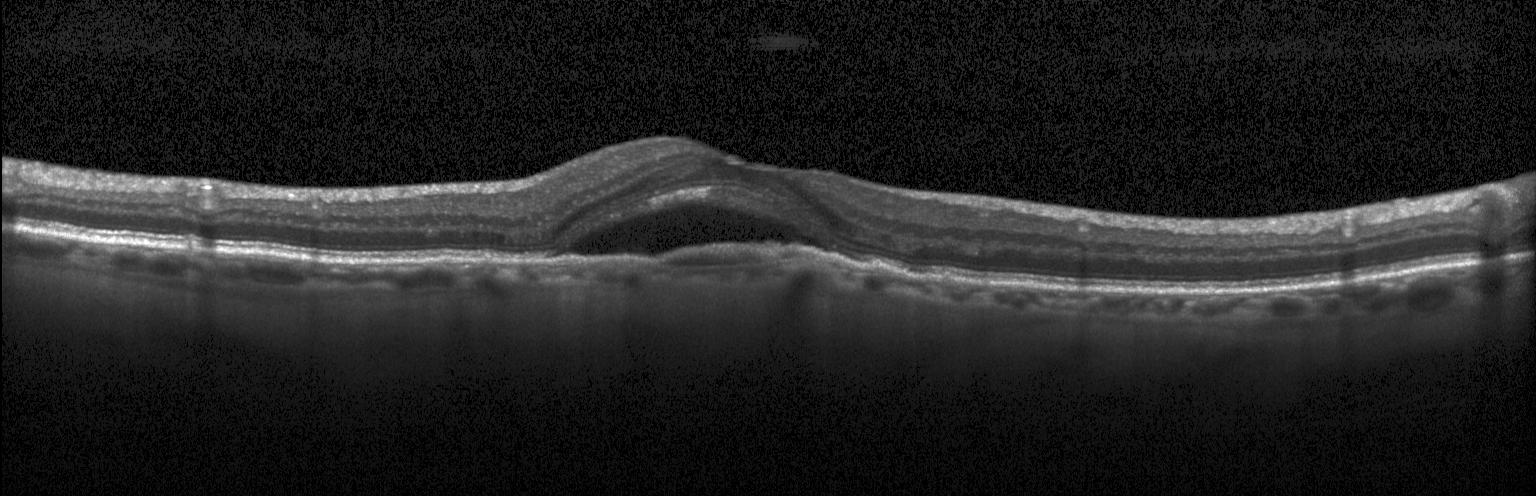 Impression: a choroidal neovascular membrane.